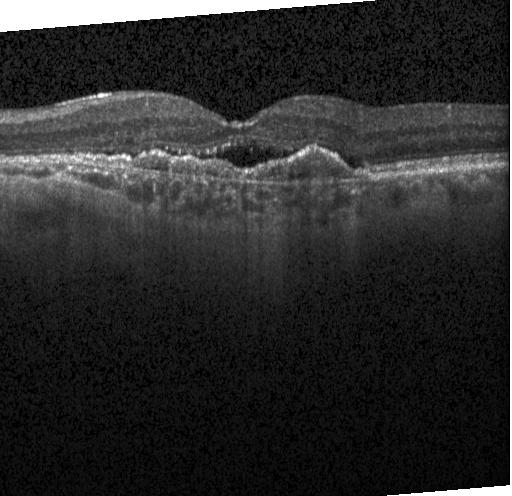
Retinal OCT B-scan · spectral-domain optical coherence tomography
Diagnosis: choroidal neovascularization.